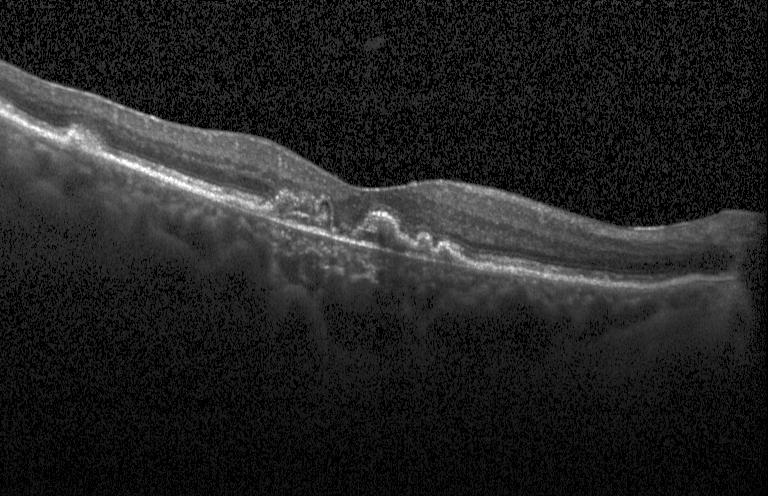 SD-OCT · retinal OCT cross-section — Macular OCT: a choroidal neovascular membrane.